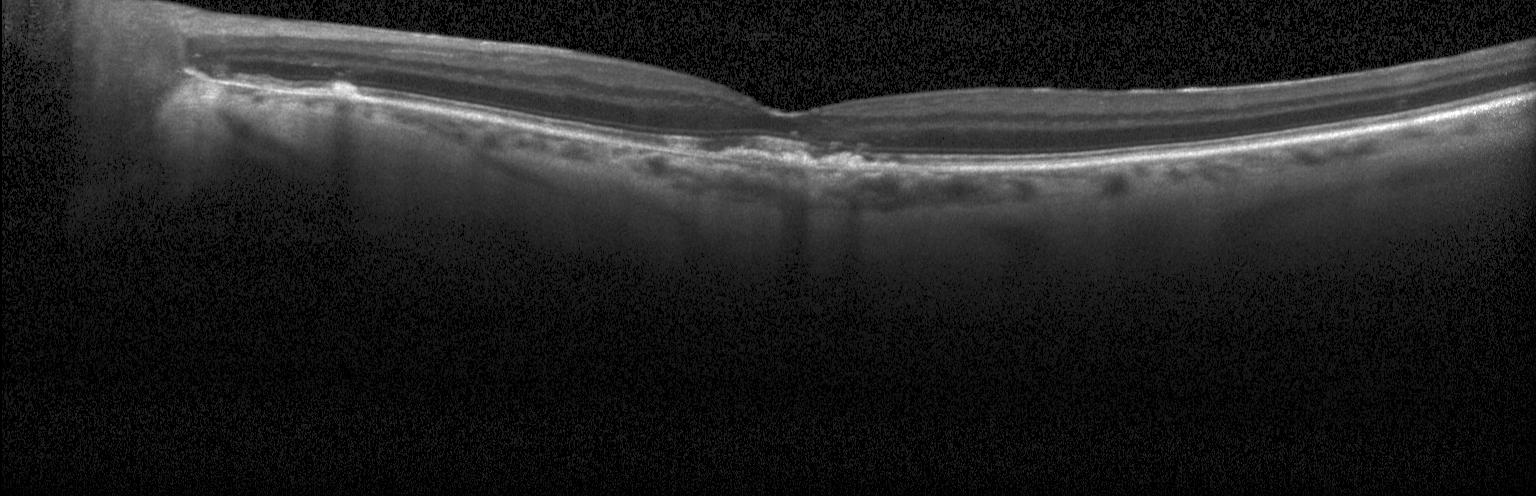
Optical coherence tomography B-scan · Heidelberg Spectralis OCT system. Diagnosis: a choroidal neovascular membrane.